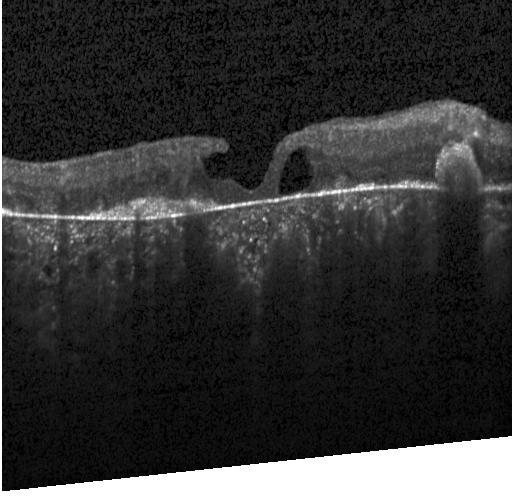 Optical coherence tomography B-scan · spectral-domain optical coherence tomography · macular scan
A choroidal neovascular membrane.